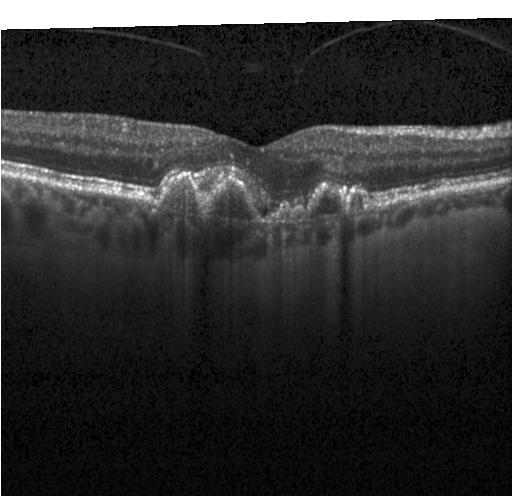
OCT B-scan.
Diagnosis: a choroidal neovascular membrane.